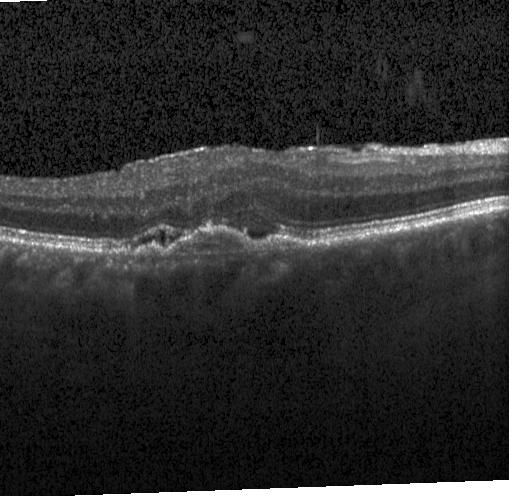

Optical coherence tomography B-scan · Heidelberg Spectralis · spectral-domain OCT · through the macula — Finding: a choroidal neovascular membrane.